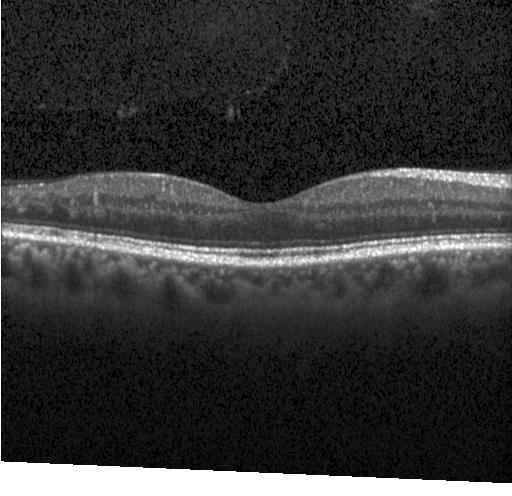 Optical coherence tomography B-scan — Finding: no choroidal neovascularization, diabetic macular edema, or drusen.